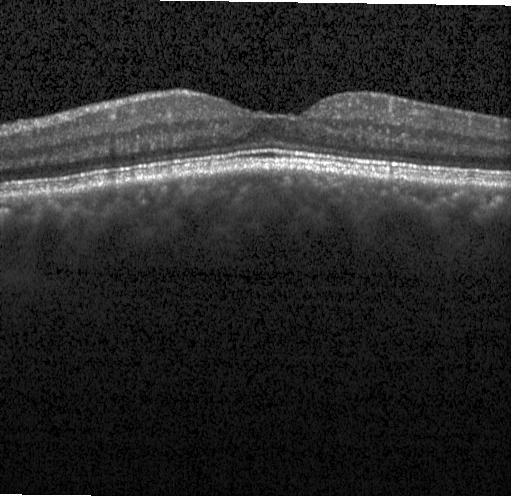

OCT B-scan.
Macular OCT: no CNV, no DME, and no drusen.